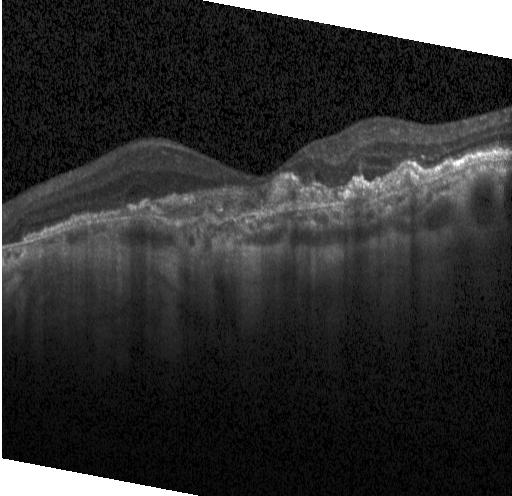 Retinal OCT cross-section — Choroidal neovascularization (CNV).